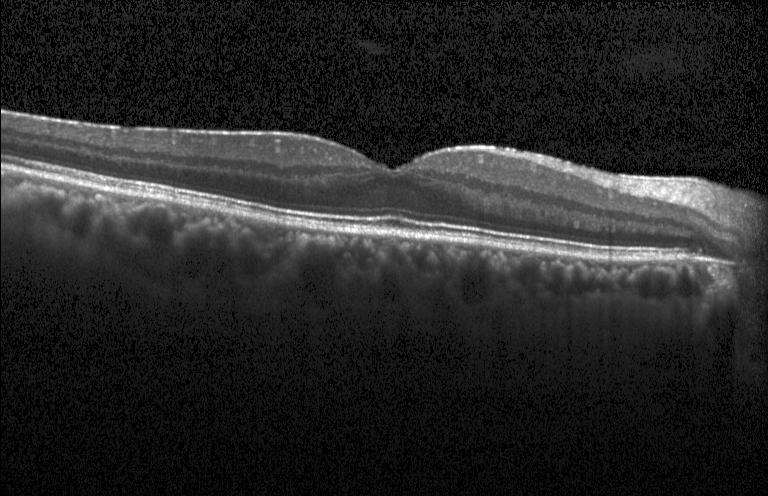
Spectral-domain OCT. Acquired on a Heidelberg Spectralis. Macular scan. Retinal OCT cross-section. Finding: no evidence of choroidal neovascularization, diabetic macular edema, or drusen.